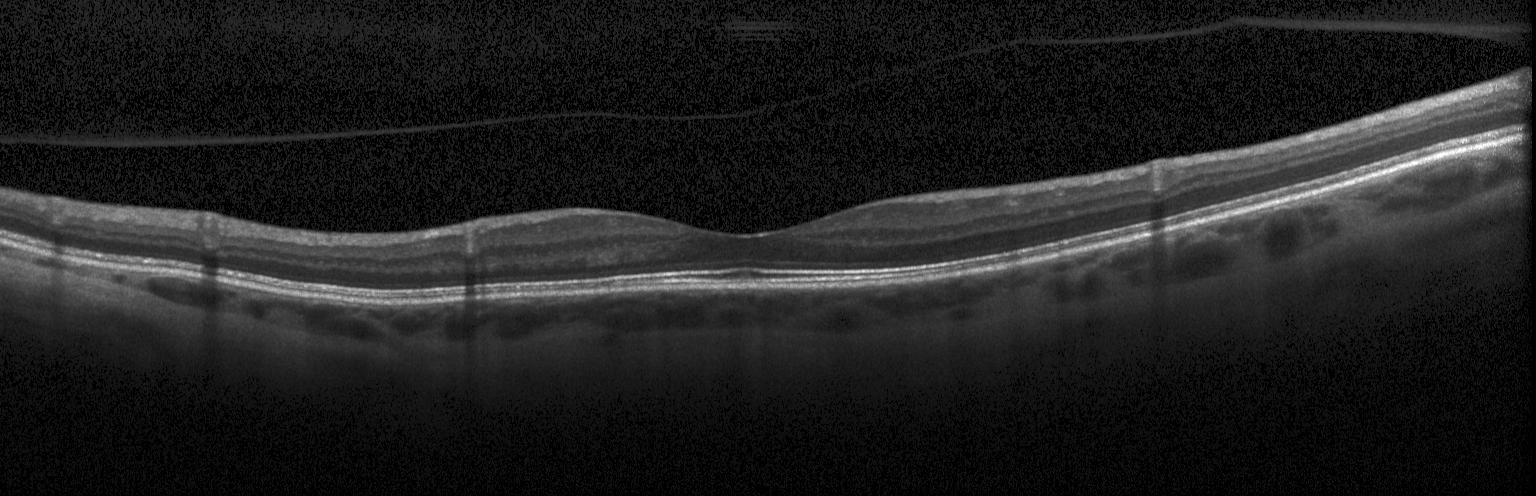
Retinal OCT B-scan.
OCT finding: neither CNV, DME, nor drusen.